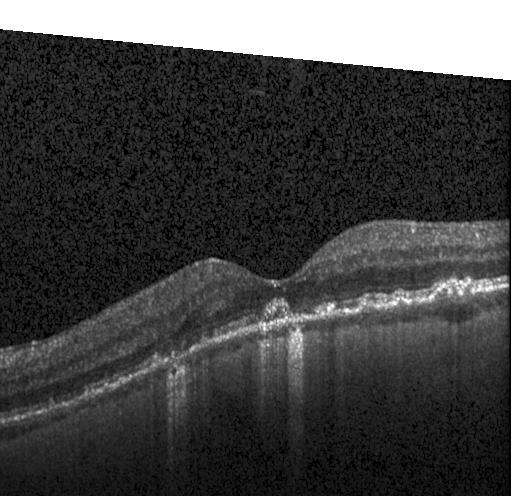 Dx: CNV.